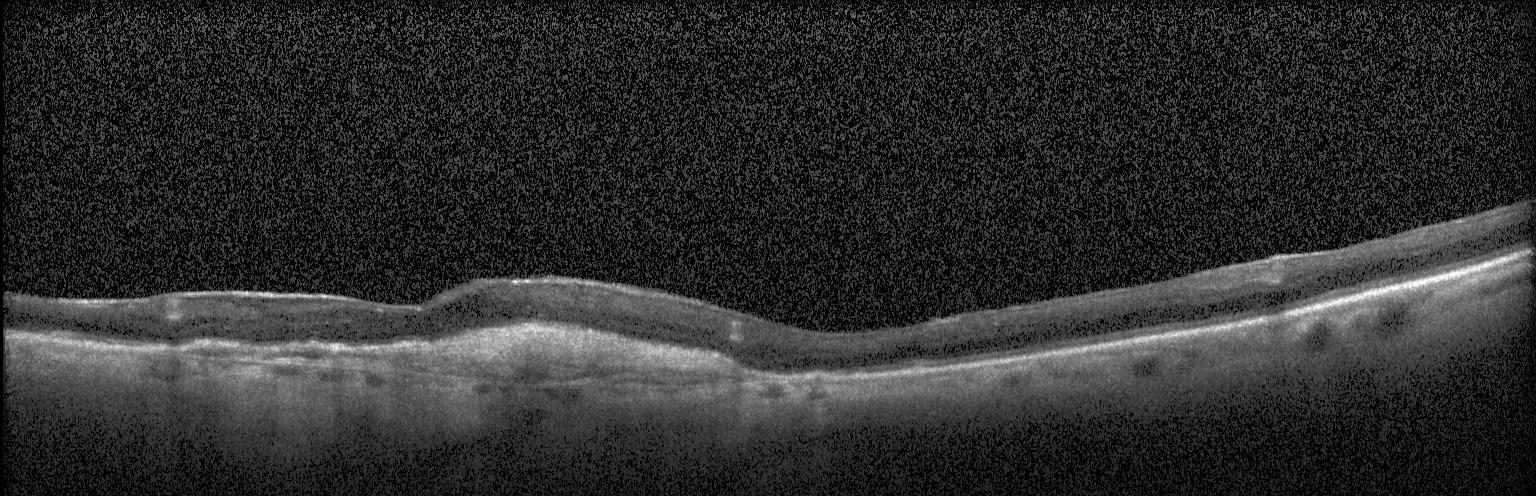 Retinal OCT B-scan. Horizontal scan through the fovea. Instrument: Heidelberg Spectralis — Impression: CNV.